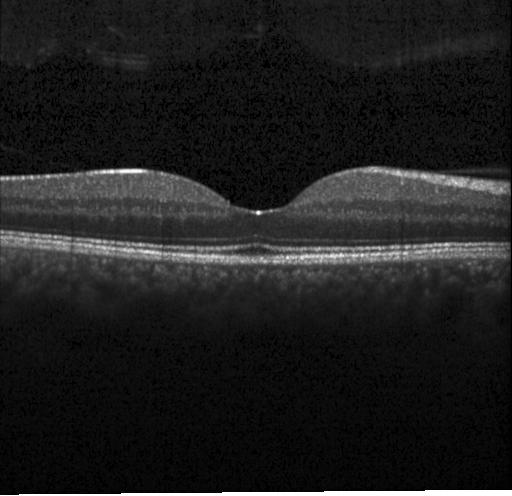
This B-scan demonstrates no evidence of choroidal neovascularization, diabetic macular edema, or drusen.